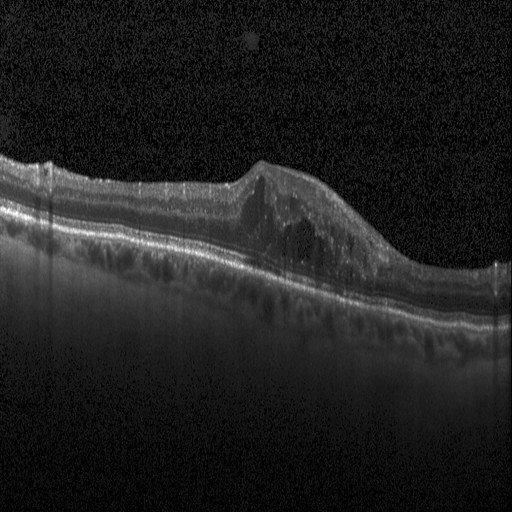

OCT B-scan. Impression: DME.